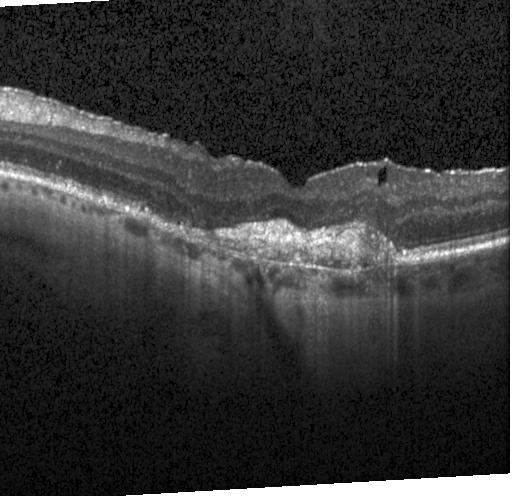
Dx: a choroidal neovascular membrane.